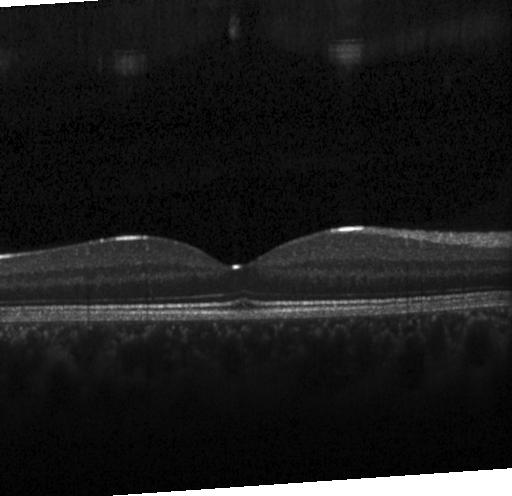 OCT line scan — The scan shows no CNV, DME, or drusen.